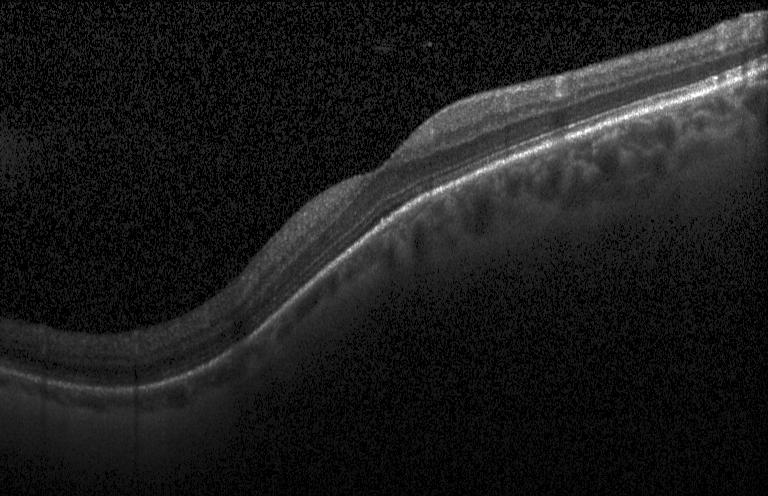

Impression: neither choroidal neovascularization, diabetic macular edema, nor drusen.